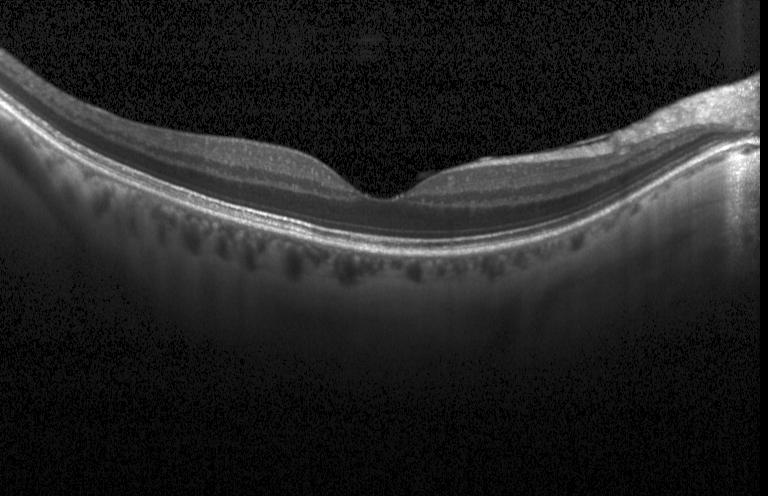
OCT scan showing neither CNV, DME, nor drusen.